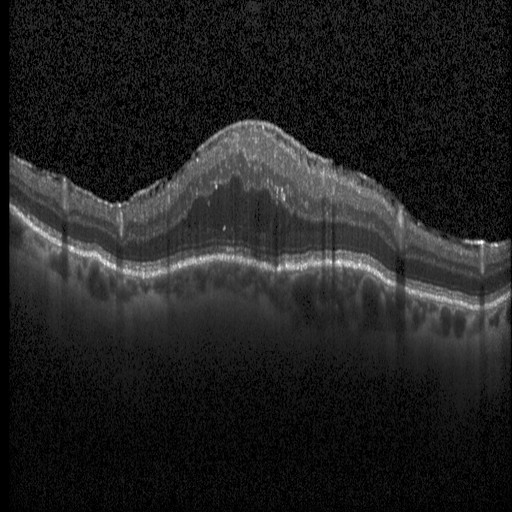 Optical coherence tomography scan.
Diagnosis: DME.